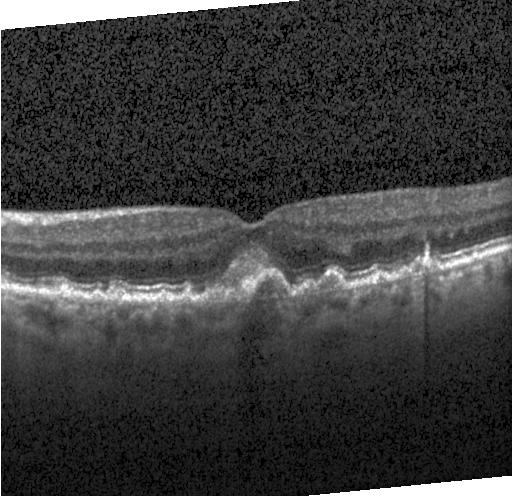
Retinal OCT cross-section showing CNV.